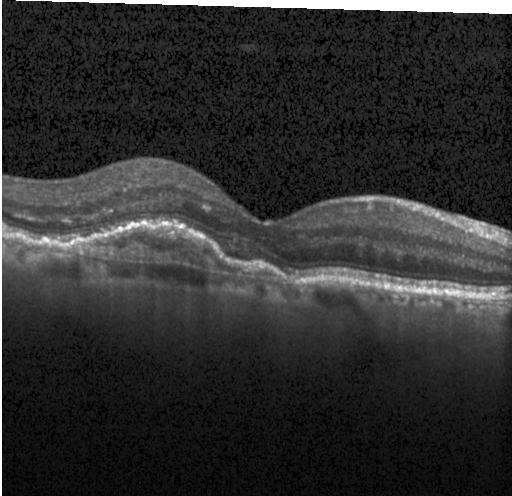 Retinal OCT cross-section showing a choroidal neovascular membrane.